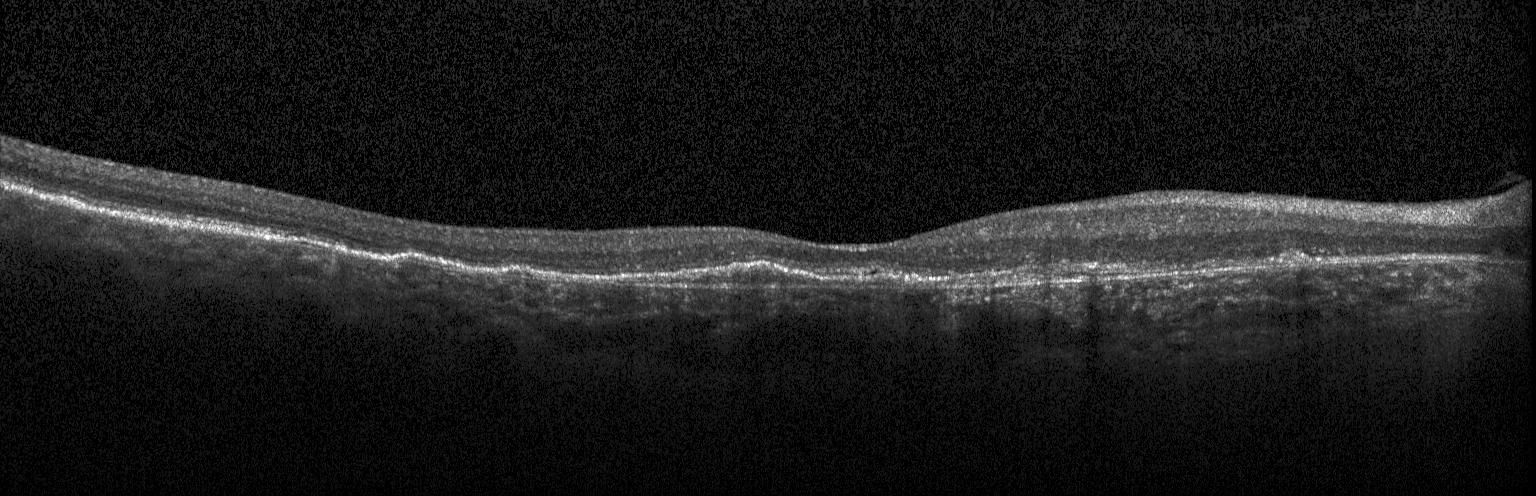 Heidelberg Spectralis, macular scan, optical coherence tomography scan — Macular OCT: a choroidal neovascular membrane.